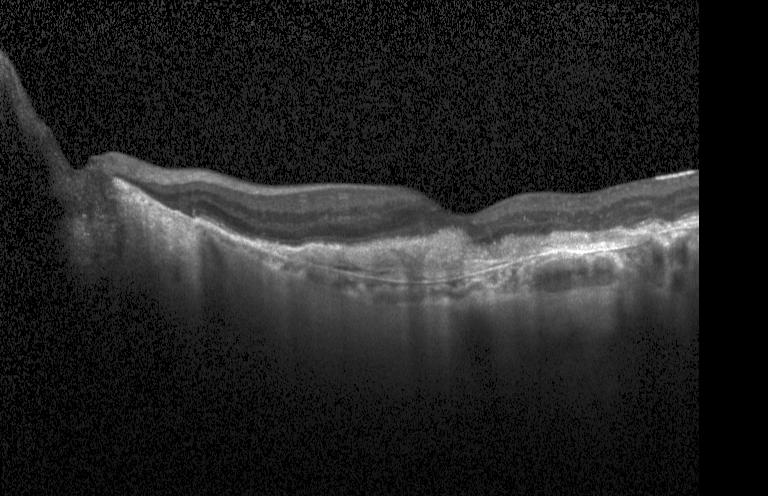

OCT scan showing CNV.